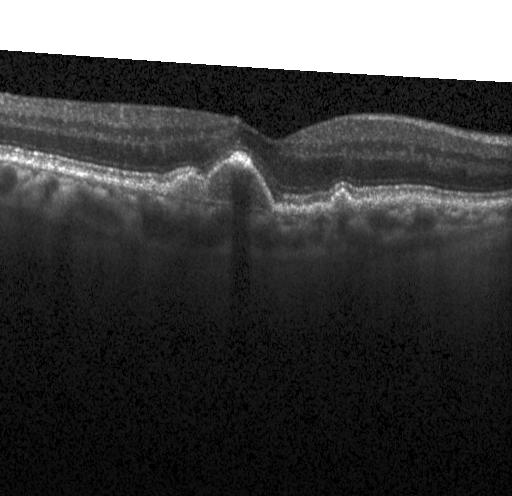

Impression: sub-RPE drusenoid deposits.